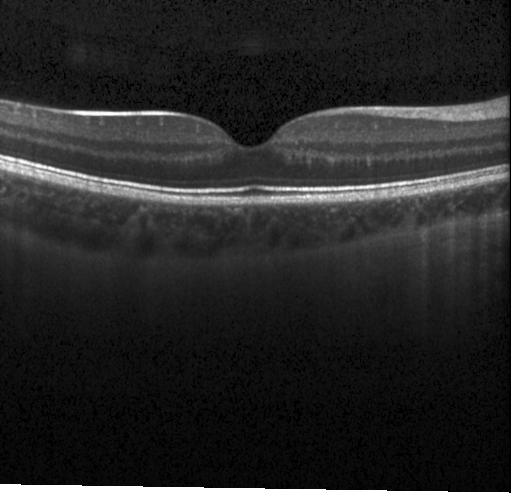 Macular OCT: no choroidal neovascularization, no diabetic macular edema, and no drusen.